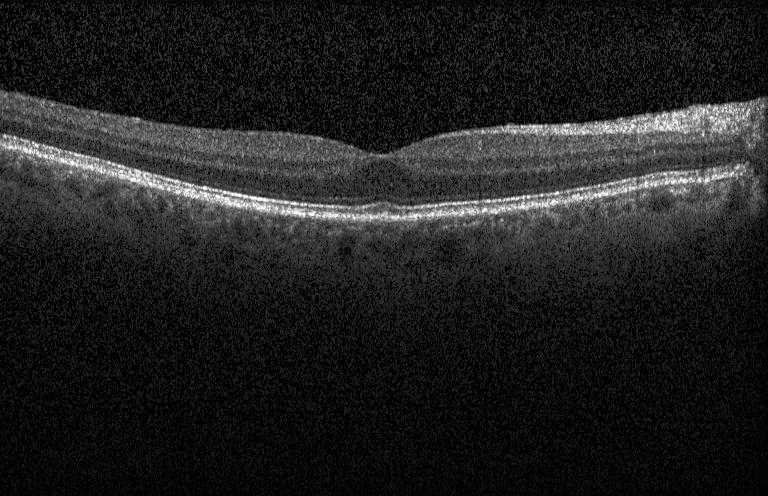

Macular OCT: no choroidal neovascularization, no diabetic macular edema, and no drusen.